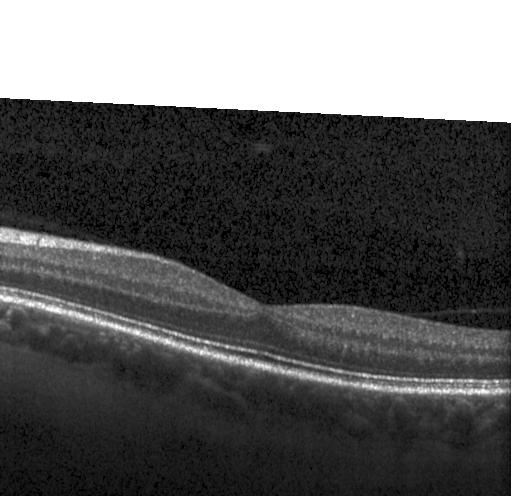
Instrument: Heidelberg Spectralis. Retinal OCT cross-section. SD-OCT. Macular OCT: no evidence of choroidal neovascularization, diabetic macular edema, or drusen.